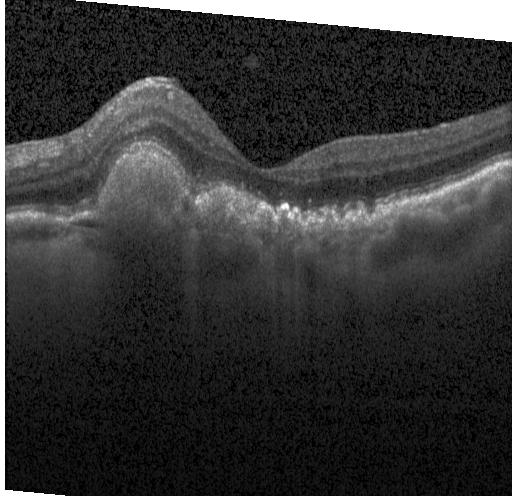 Assessment: a choroidal neovascular membrane.